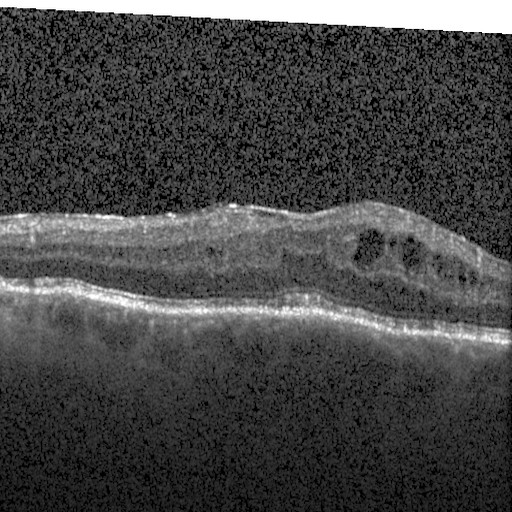
Retinal OCT B-scan; macular scan
Assessment: diabetic macular edema.